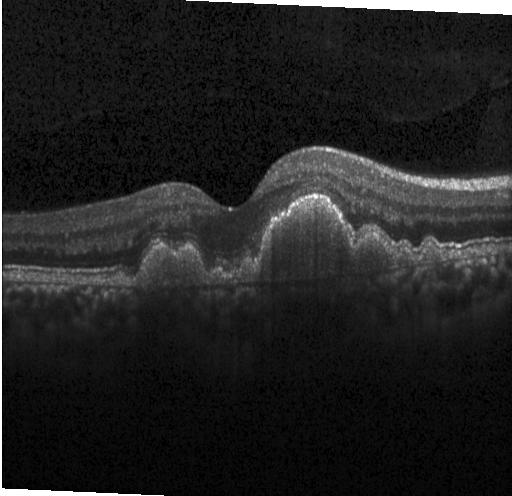
Optical coherence tomography scan.
Drusen.